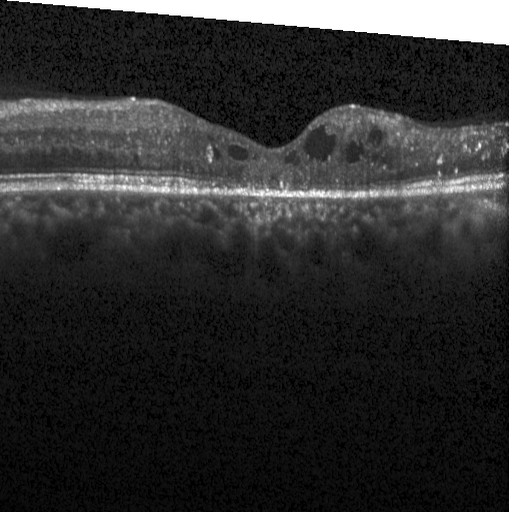 Diagnosis: diabetic macular edema (DME).